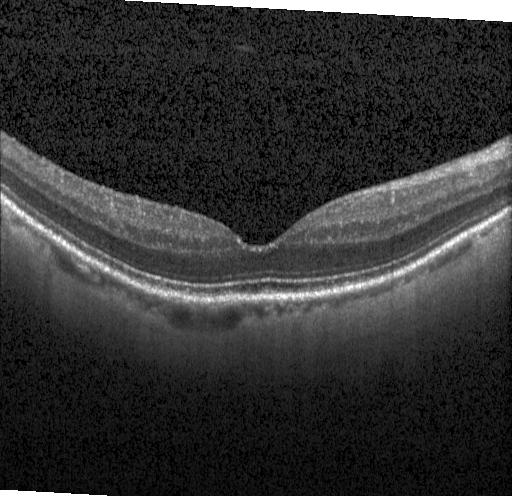

Macular OCT: no evidence of CNV, DME, or drusen.